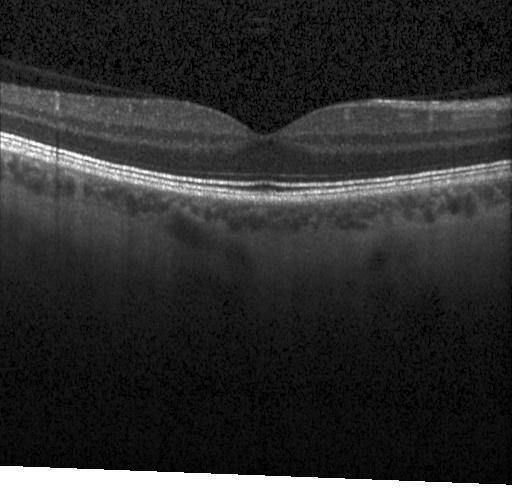
OCT B-scan, macular scan.
The scan shows neither CNV, DME, nor drusen.